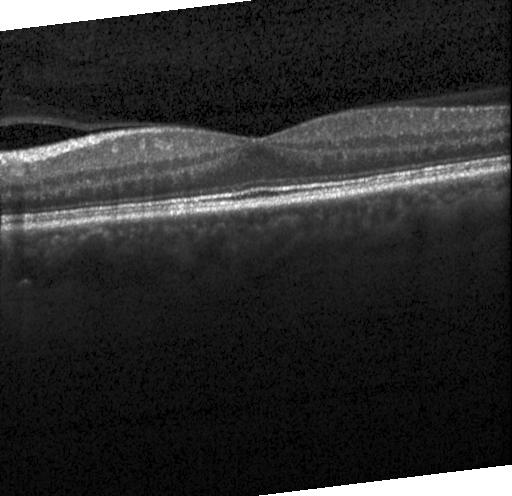

OCT B-scan
Impression: no choroidal neovascularization, diabetic macular edema, or drusen.